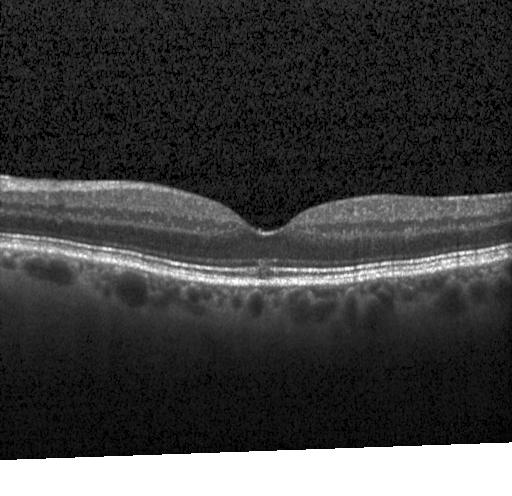

Diagnosis: no evidence of choroidal neovascularization, diabetic macular edema, or drusen.